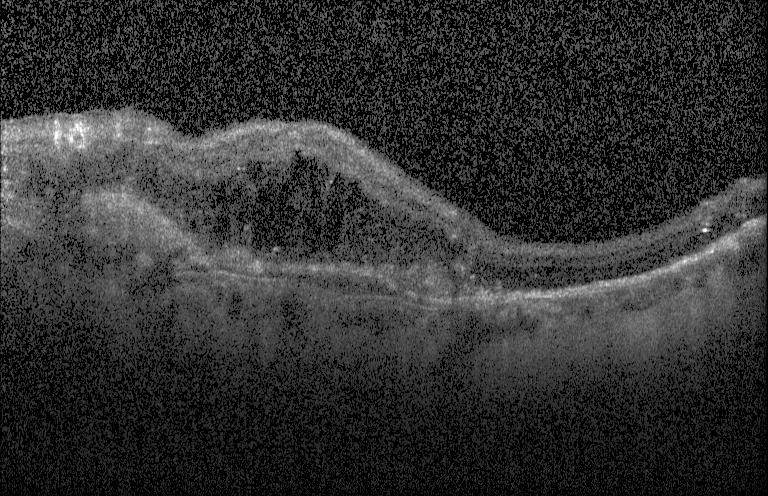 Optical coherence tomography scan · spectral-domain optical coherence tomography · horizontal scan through the fovea.
This B-scan demonstrates a choroidal neovascular membrane.